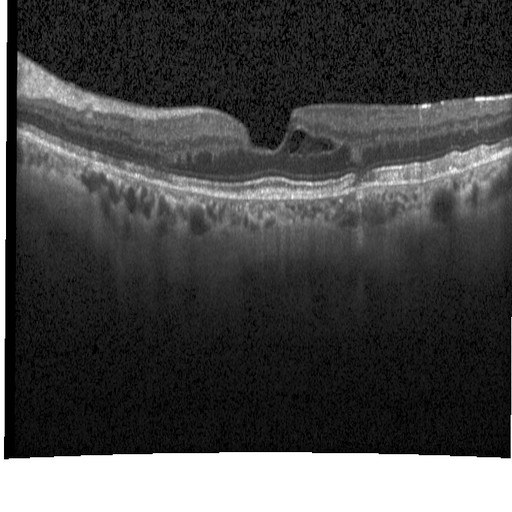 Spectral-domain optical coherence tomography. Heidelberg Spectralis OCT system. Through the macula. OCT B-scan. This B-scan demonstrates diabetic macular edema (DME).